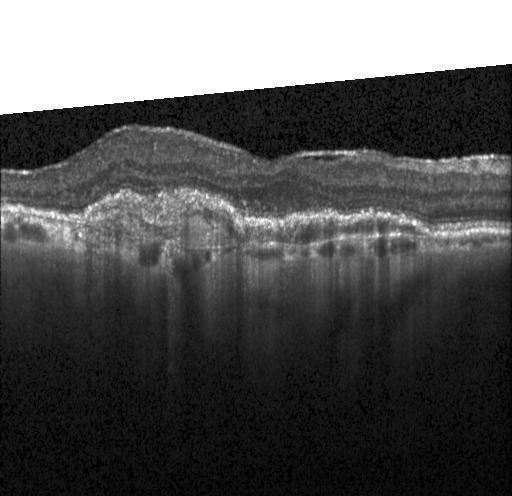
Centered on the fovea · OCT line scan.
Impression: choroidal neovascularization (CNV).